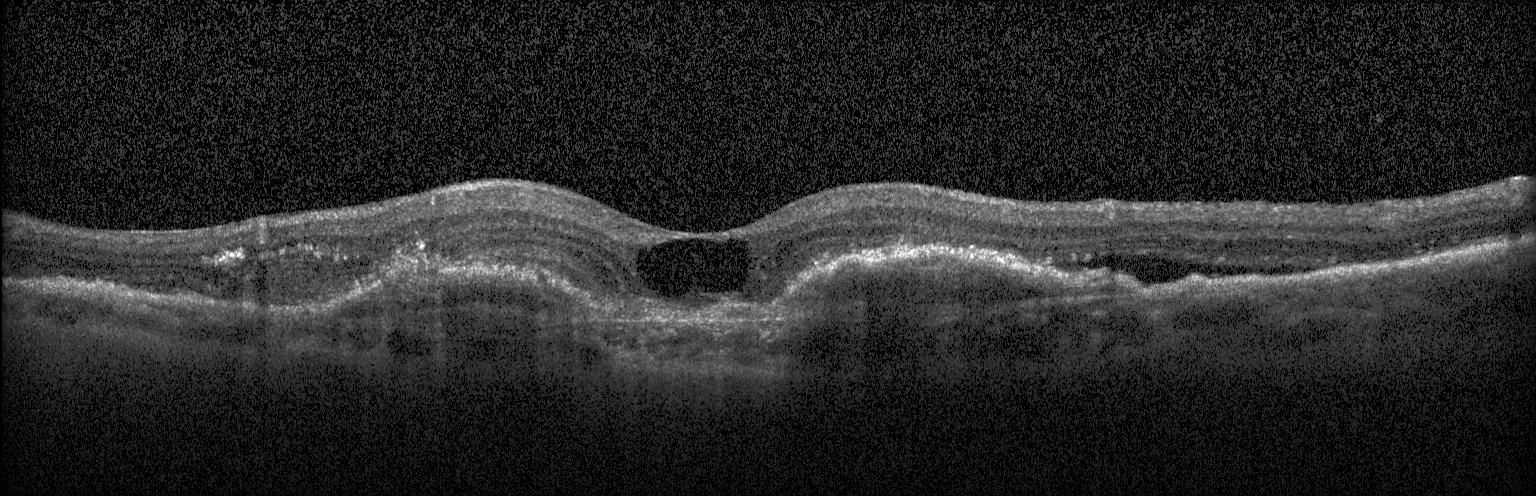
Impression: a choroidal neovascular membrane.